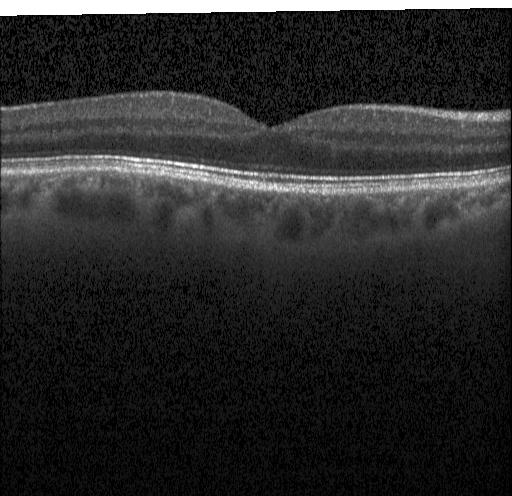

Assessment: no CNV, DME, or drusen.